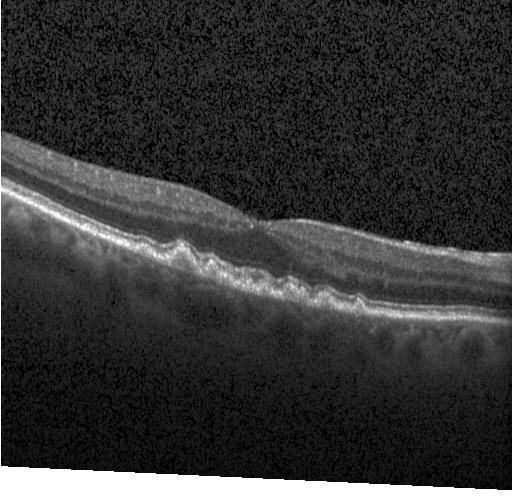
Horizontal scan through the fovea · Heidelberg Spectralis · OCT B-scan.
Dx: multiple drusen.